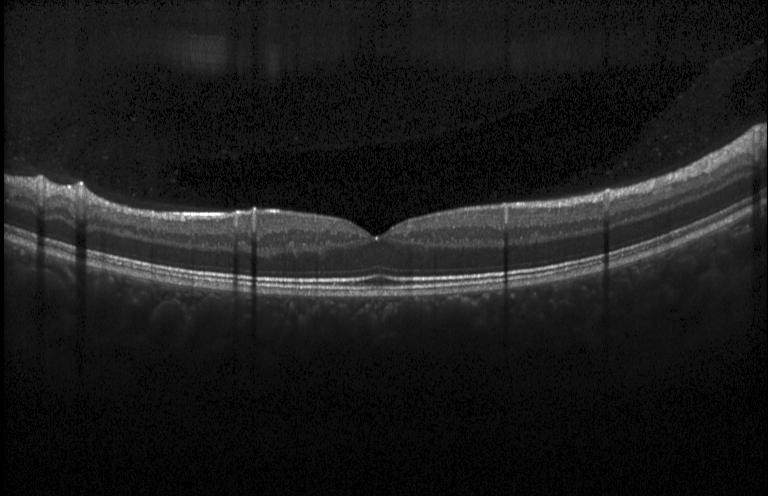
Heidelberg Spectralis; spectral-domain OCT; retinal OCT cross-section.
Diagnosis: neither CNV, DME, nor drusen.